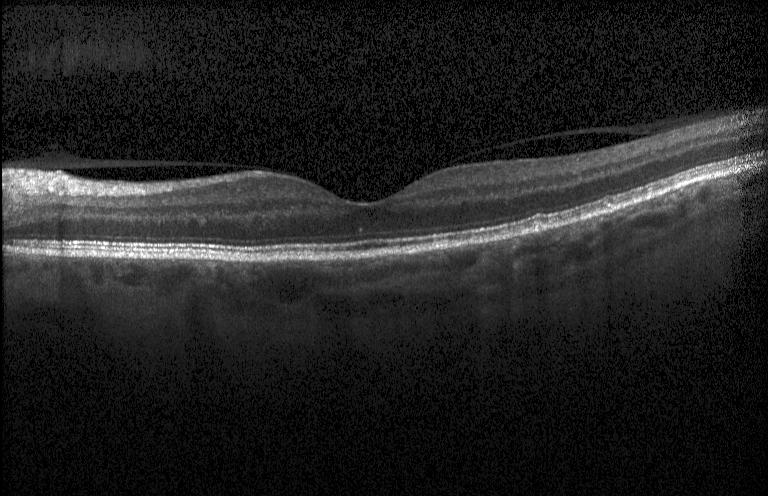
OCT B-scan, spectral-domain optical coherence tomography, horizontal scan through the fovea, Heidelberg Spectralis
Assessment: sub-RPE drusenoid deposits.